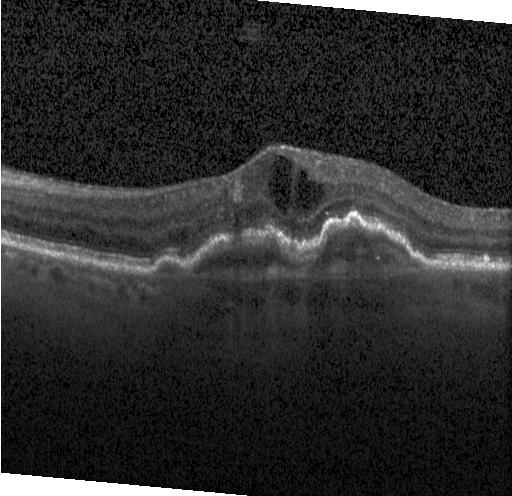

Acquired on a Heidelberg Spectralis. OCT line scan
Impression: CNV.